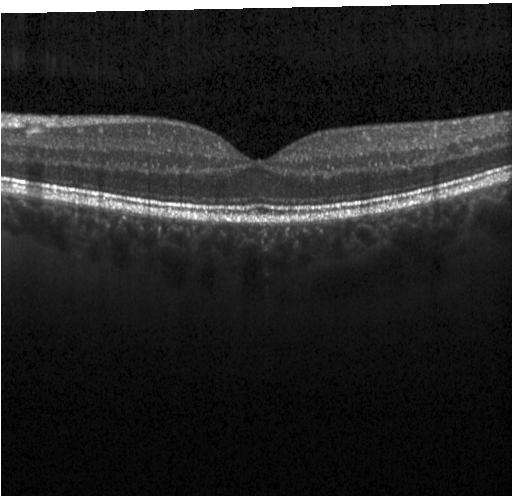 Macular OCT: no CNV, DME, or drusen.